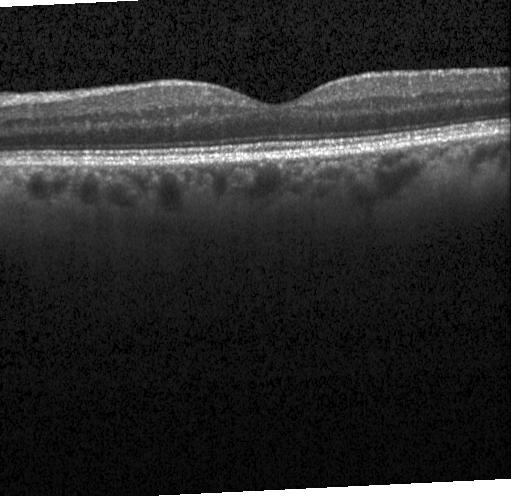 No evidence of CNV, DME, or drusen.